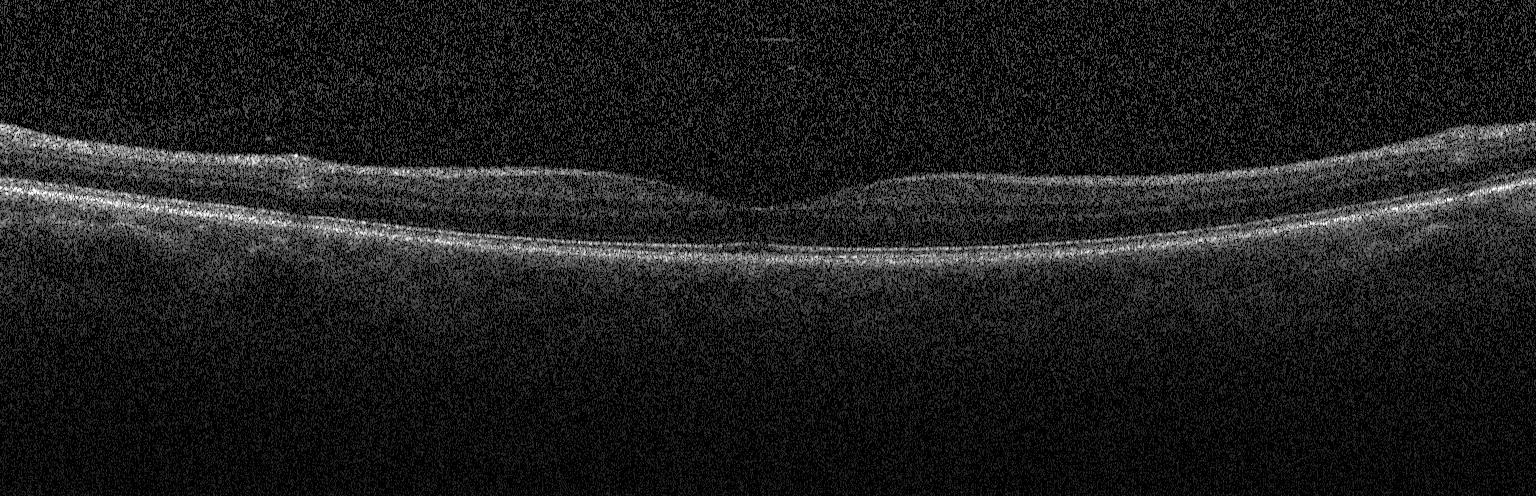

Impression: no CNV, no DME, and no drusen.